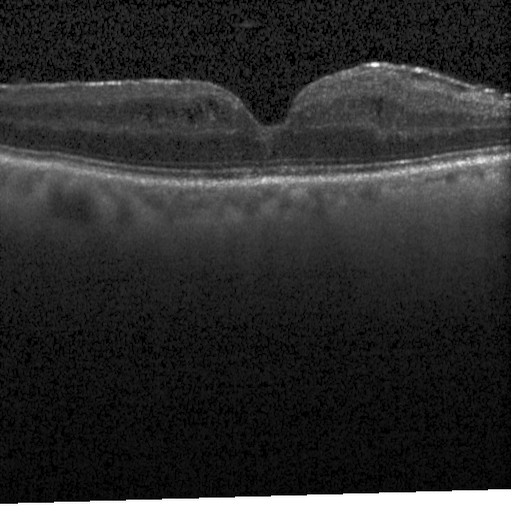

Spectral-domain OCT, retinal OCT cross-section, acquired on a Heidelberg Spectralis
Dx: DME.